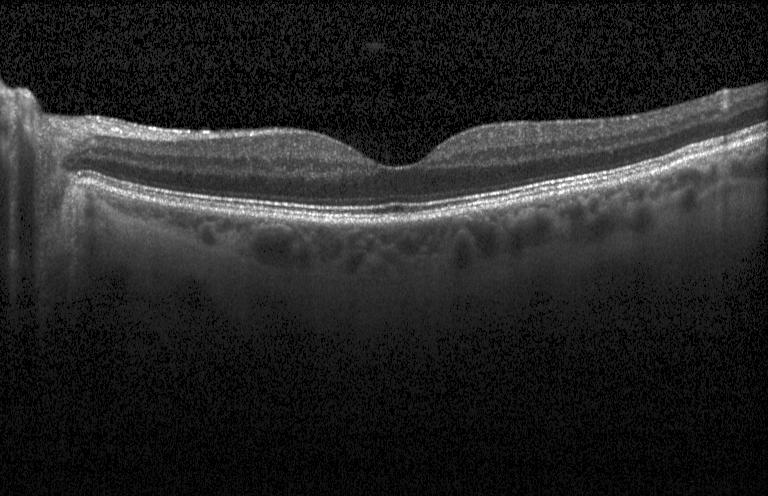
Macular OCT: no choroidal neovascularization, diabetic macular edema, or drusen.